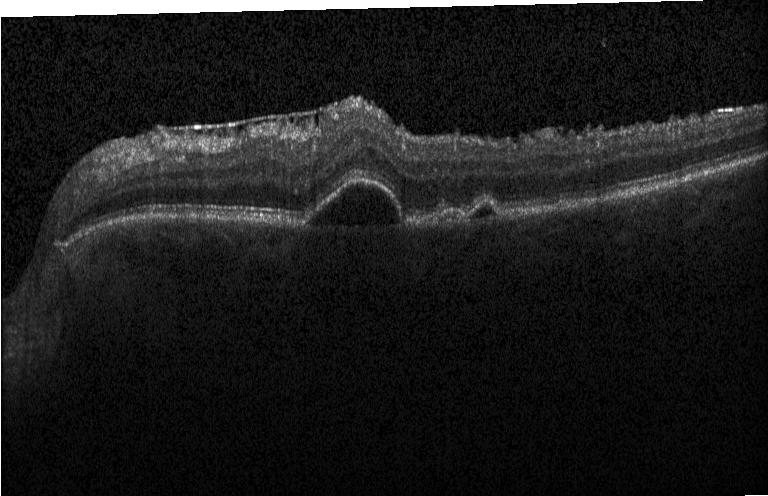 OCT B-scan; Heidelberg Spectralis OCT system
A choroidal neovascular membrane.